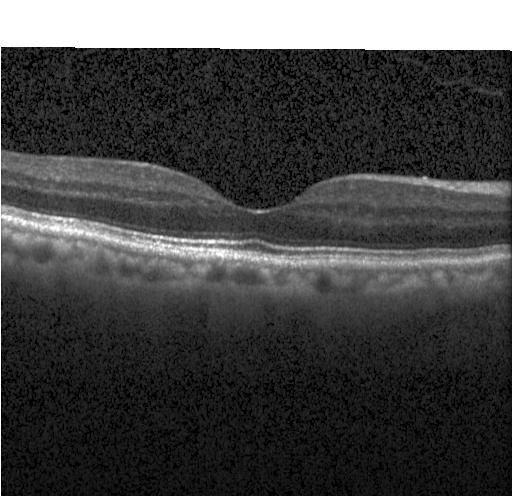 Optical coherence tomography B-scan, SD-OCT
This B-scan demonstrates neither choroidal neovascularization, diabetic macular edema, nor drusen.